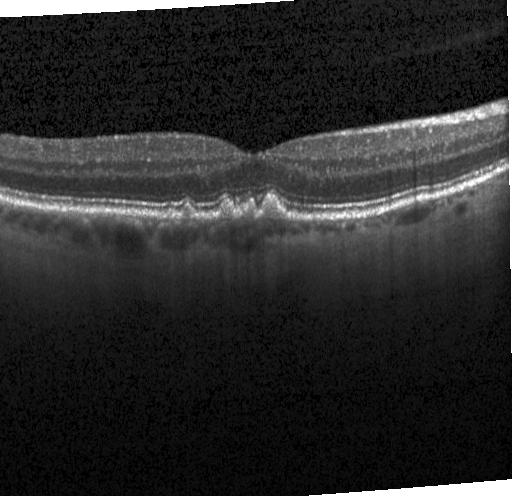

Diagnosis: multiple drusen.